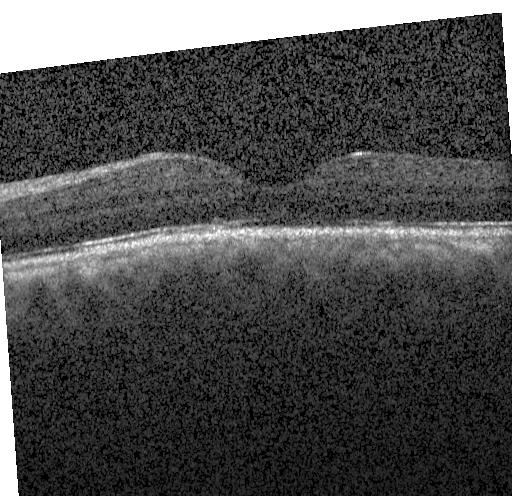
Through the macula, optical coherence tomography scan — Assessment: no CNV, no DME, and no drusen.